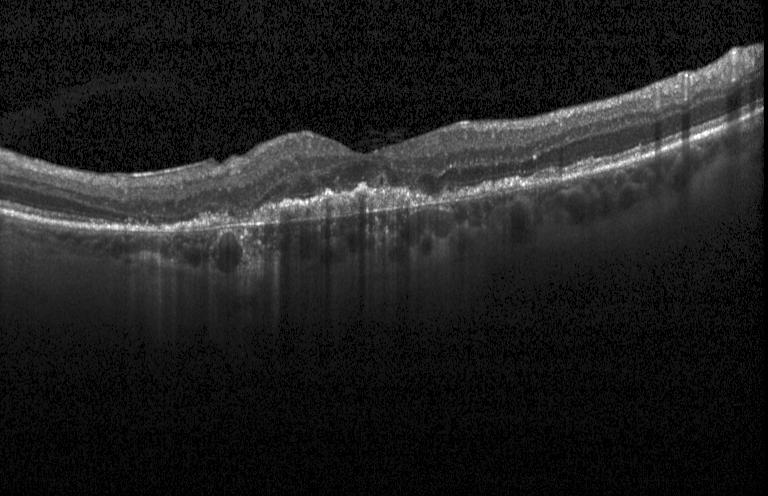 Assessment: CNV.